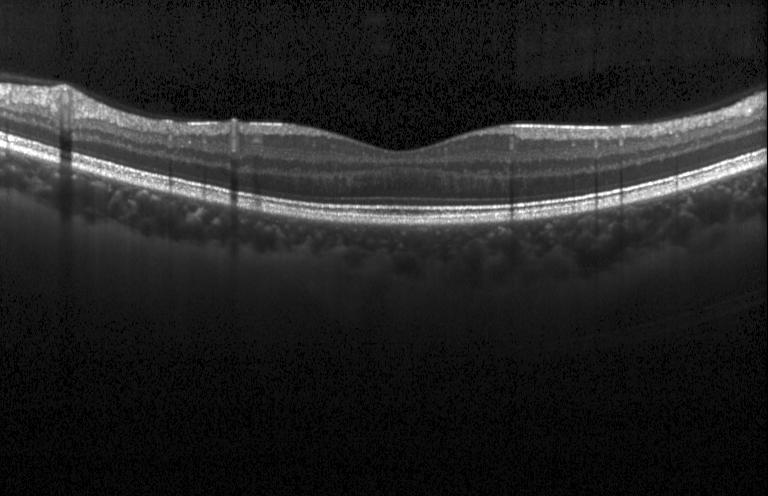

Centered on the fovea, Heidelberg Spectralis, OCT B-scan, spectral-domain OCT. Diagnosis: no choroidal neovascularization, no diabetic macular edema, and no drusen.